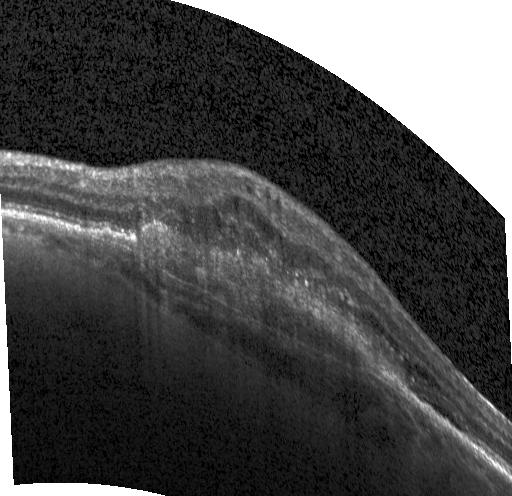
OCT B-scan, instrument: Heidelberg Spectralis
Dx: CNV.